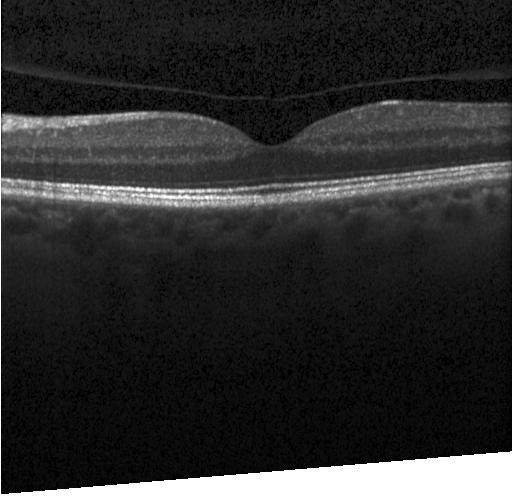

Optical coherence tomography scan. Macular scan — Impression: no evidence of choroidal neovascularization, diabetic macular edema, or drusen.